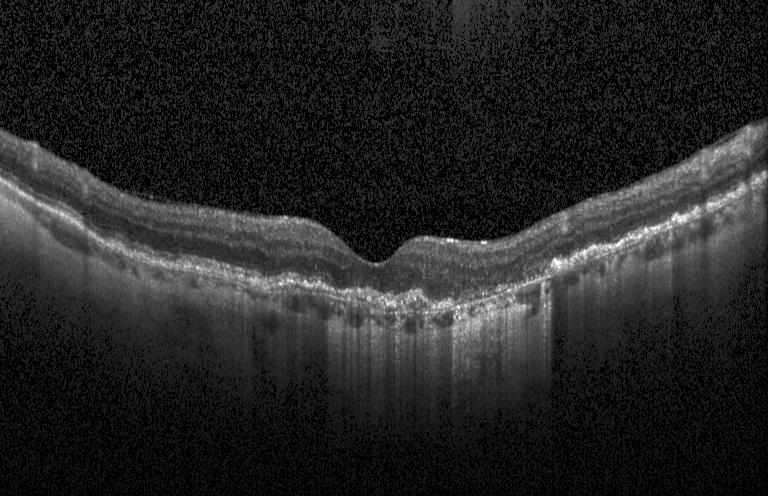 Optical coherence tomography B-scan, spectral-domain OCT.
A choroidal neovascular membrane.